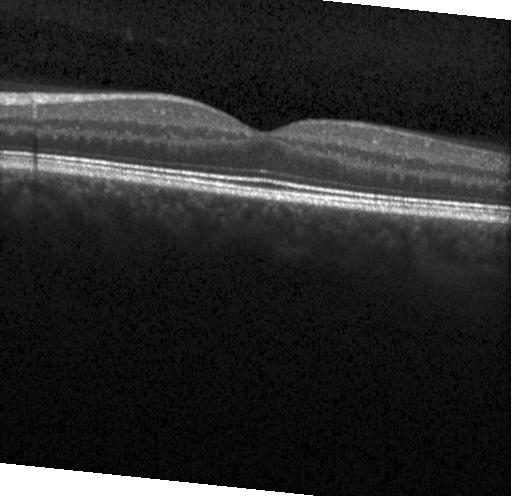

Spectral-domain optical coherence tomography, OCT B-scan
The scan shows neither choroidal neovascularization, diabetic macular edema, nor drusen.